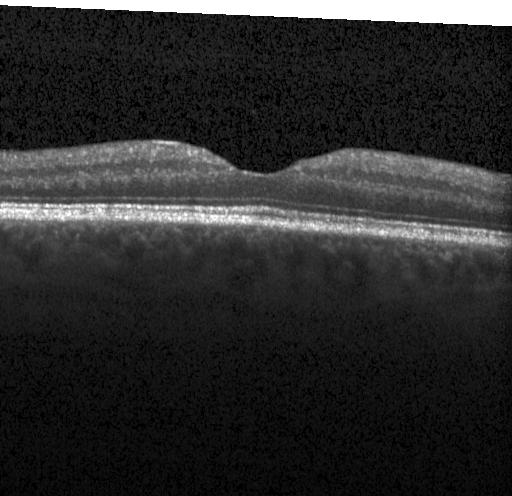 Finding: no choroidal neovascularization, diabetic macular edema, or drusen.